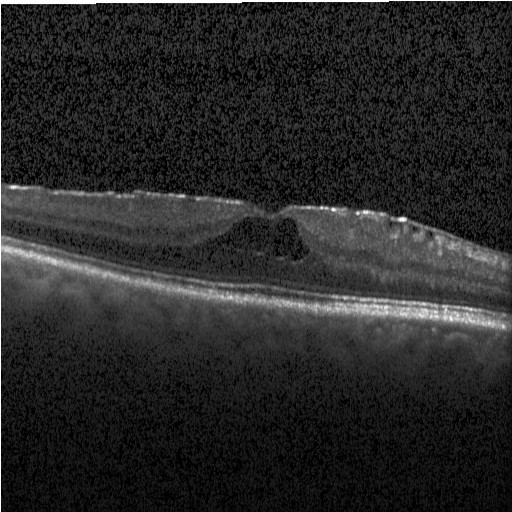

Impression: diabetic macular edema (DME).